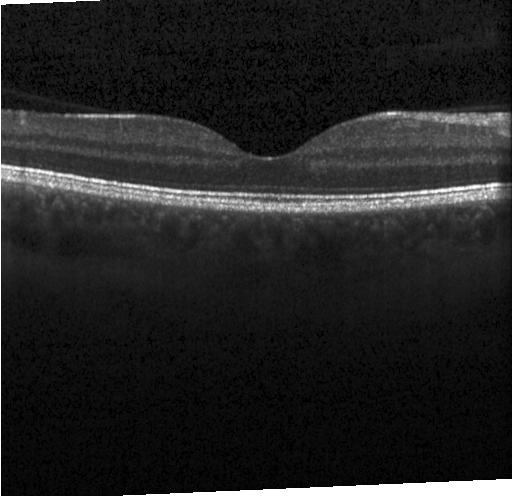 Optical coherence tomography scan, spectral-domain OCT
Dx: no evidence of choroidal neovascularization, diabetic macular edema, or drusen.